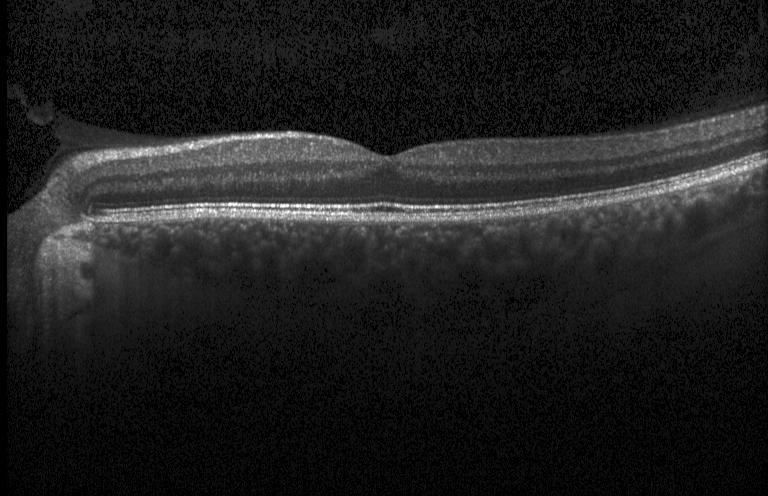 Macular scan; retinal OCT cross-section; SD-OCT.
OCT finding: no CNV, no DME, and no drusen.